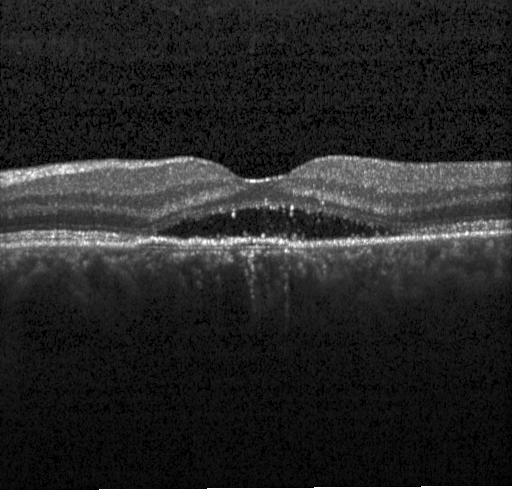

Impression: choroidal neovascularization.